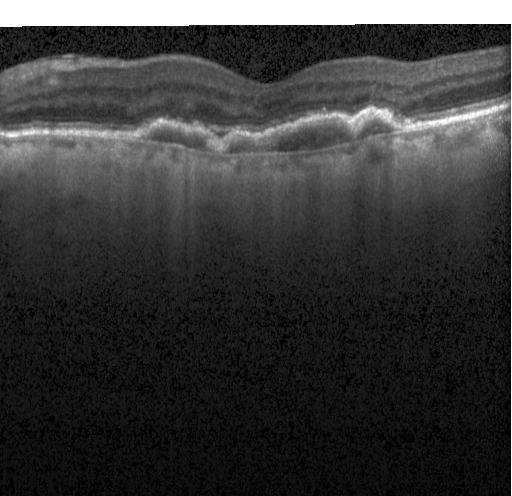
This B-scan demonstrates a choroidal neovascular membrane.